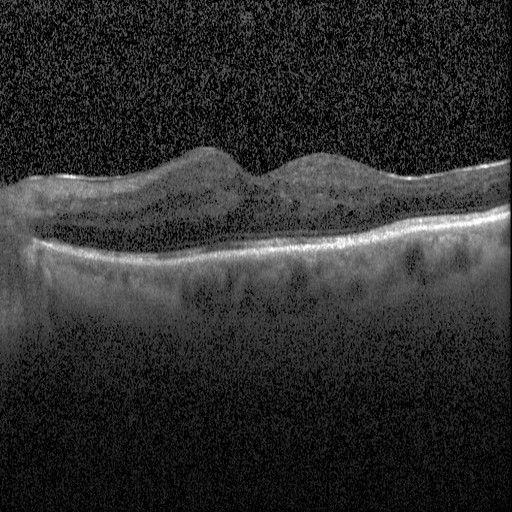 Heidelberg Spectralis, spectral-domain optical coherence tomography, retinal OCT cross-section.
Macular OCT: DME.